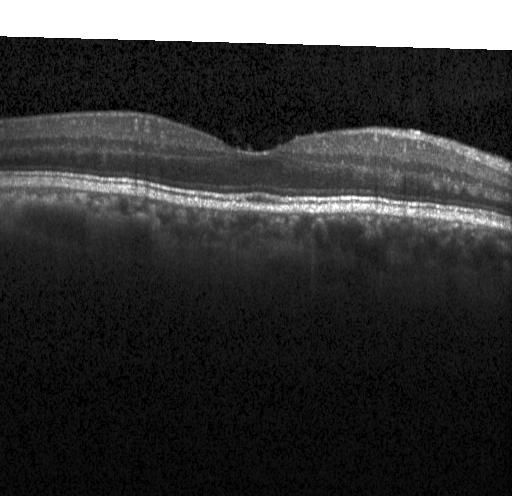 OCT line scan; instrument: Heidelberg Spectralis; spectral-domain optical coherence tomography; fovea-centered. The scan shows neither choroidal neovascularization, diabetic macular edema, nor drusen.